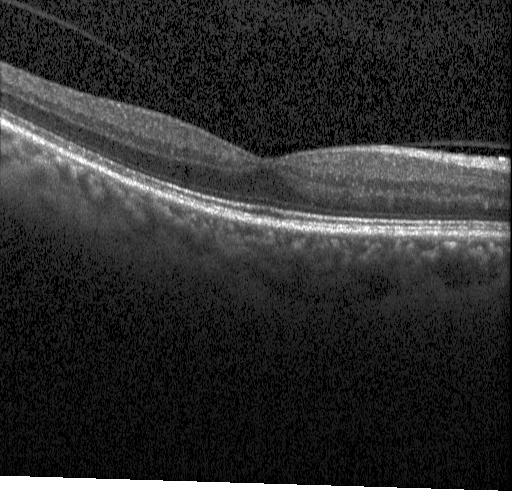

OCT B-scan · spectral-domain optical coherence tomography. Impression: no evidence of choroidal neovascularization, diabetic macular edema, or drusen.